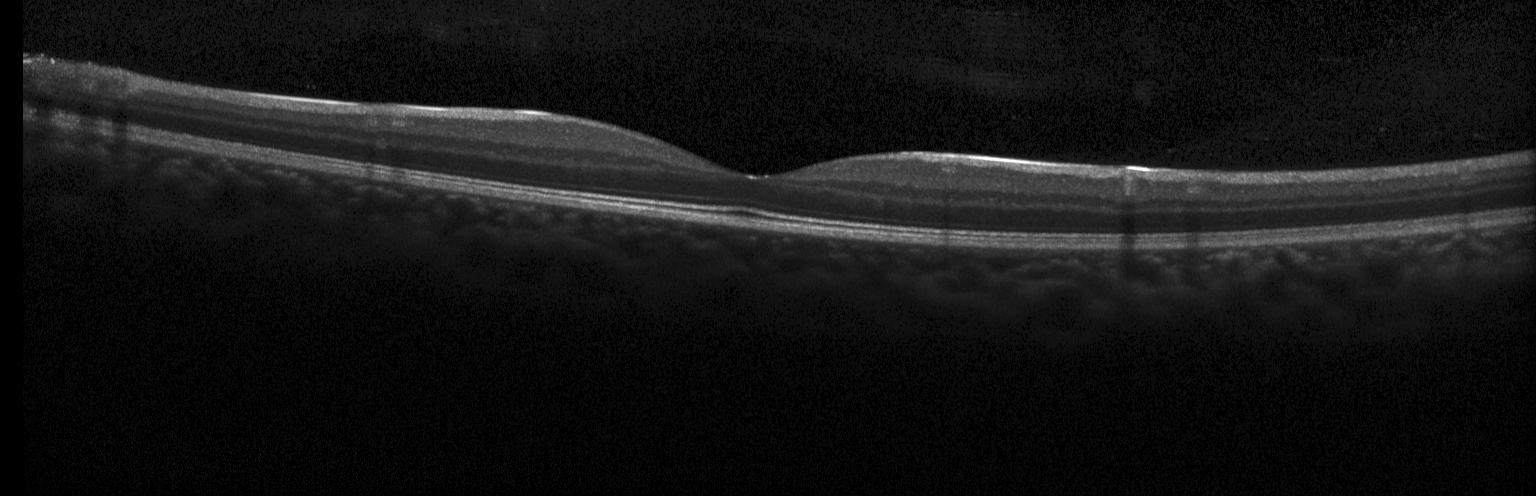 Dx: neither choroidal neovascularization, diabetic macular edema, nor drusen.